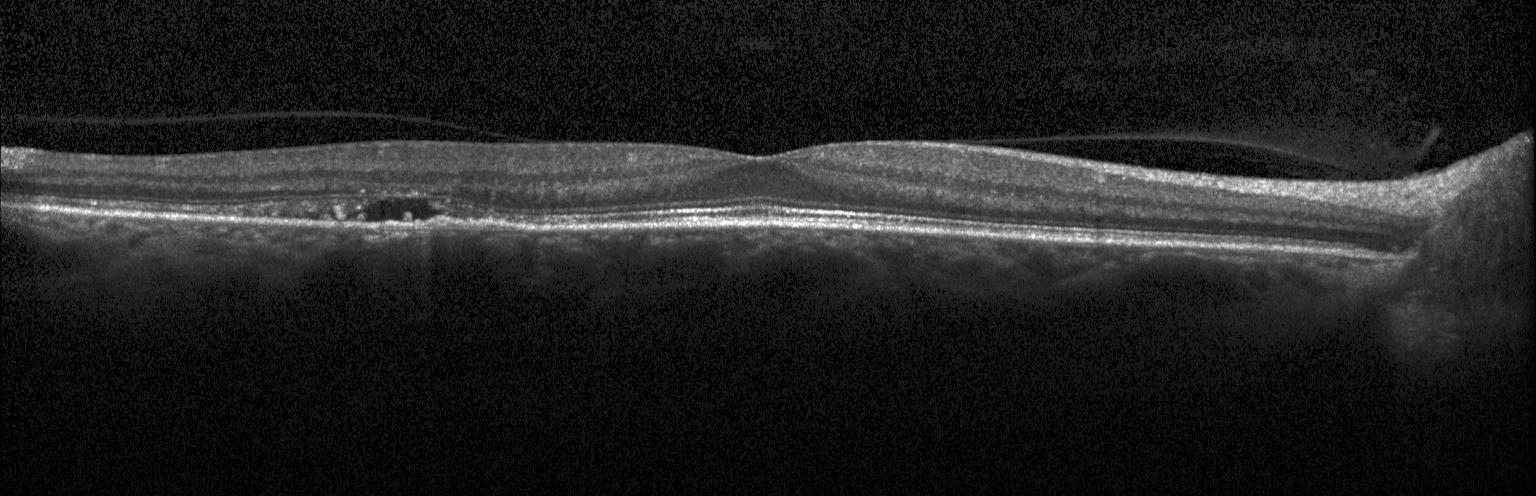 Optical coherence tomography scan; horizontal scan through the fovea.
Diagnosis: choroidal neovascularization (CNV).